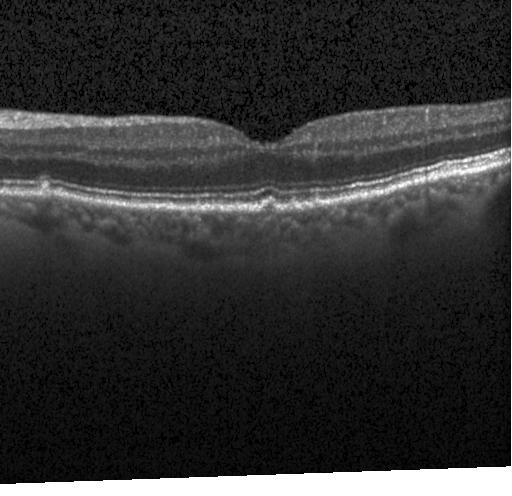 Sub-RPE drusenoid deposits.